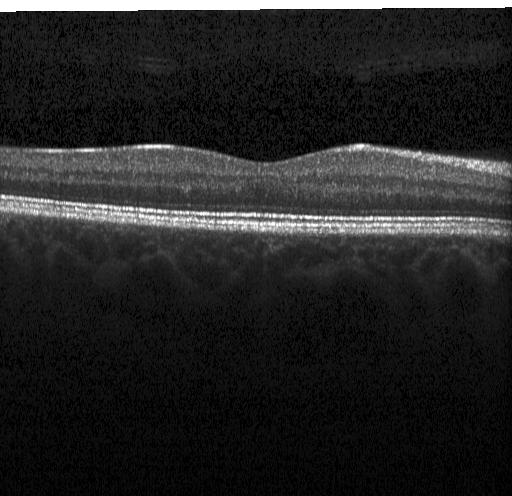
Instrument: Heidelberg Spectralis; optical coherence tomography scan — Finding: neither choroidal neovascularization, diabetic macular edema, nor drusen.